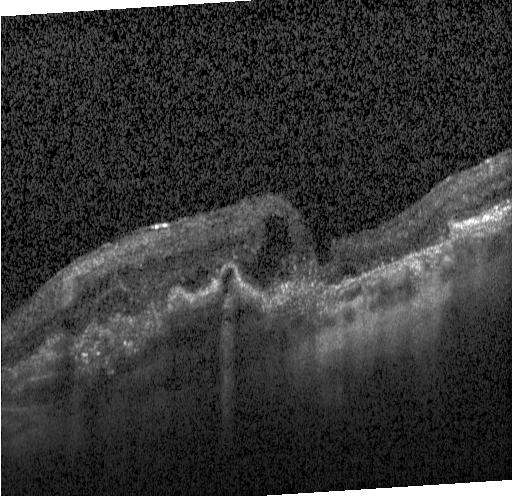 Finding: a choroidal neovascular membrane.